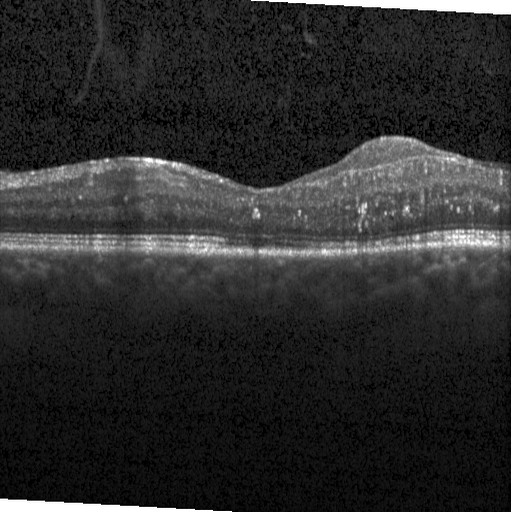
Retinal OCT B-scan. Impression: DME.